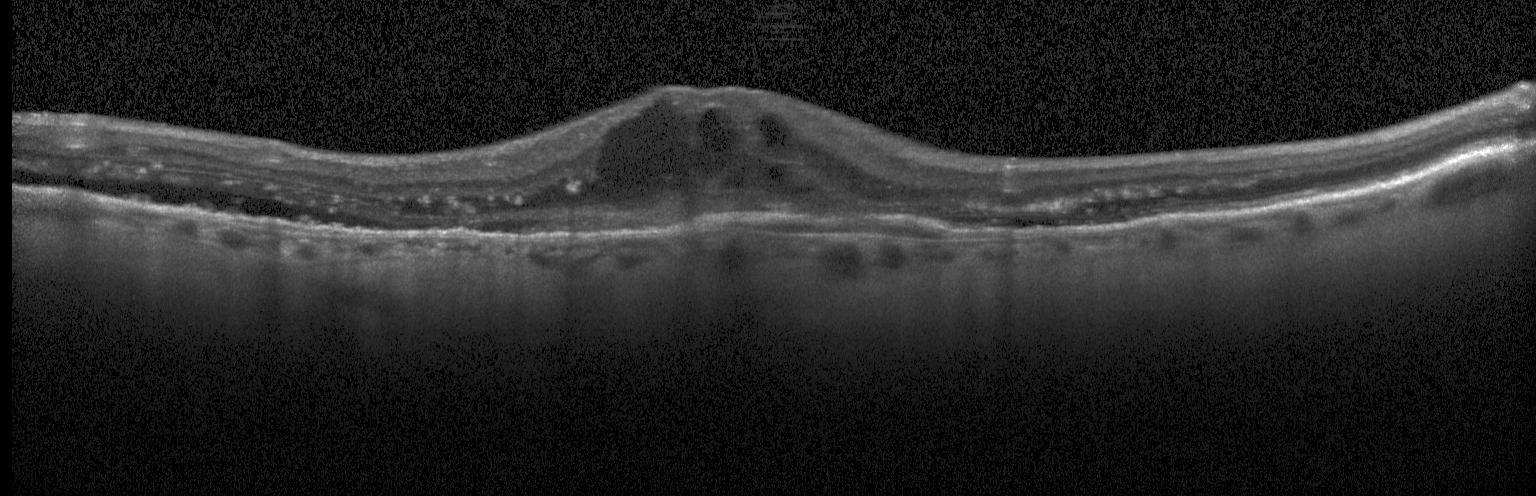 OCT line scan. Impression: choroidal neovascularization.